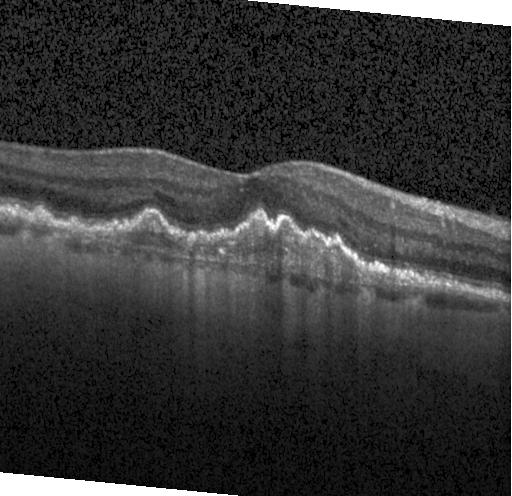
Acquired on a Heidelberg Spectralis · retinal OCT cross-section · macular scan
Finding: CNV.